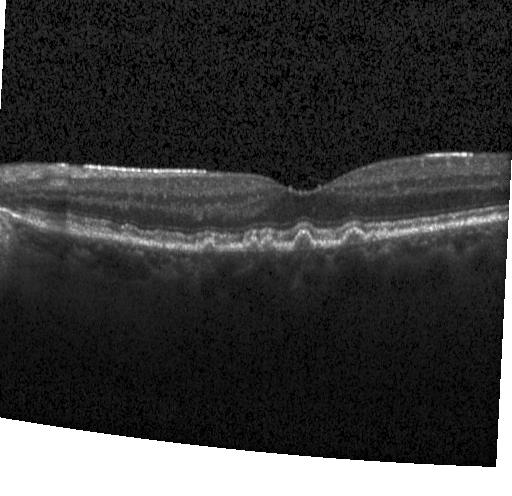
Optical coherence tomography B-scan · Heidelberg Spectralis.
Impression: multiple drusen.